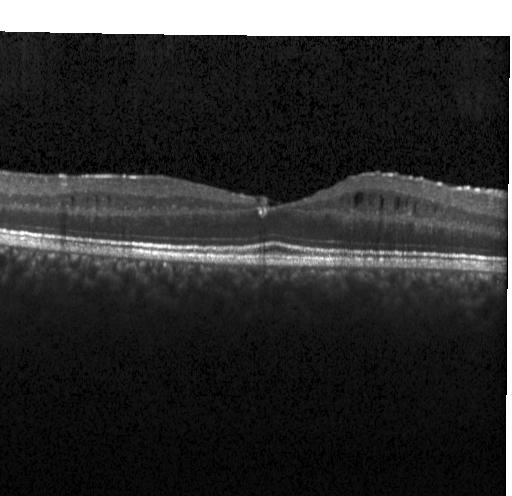
Spectral-domain OCT; instrument: Heidelberg Spectralis; optical coherence tomography scan.
This B-scan demonstrates diabetic macular edema.